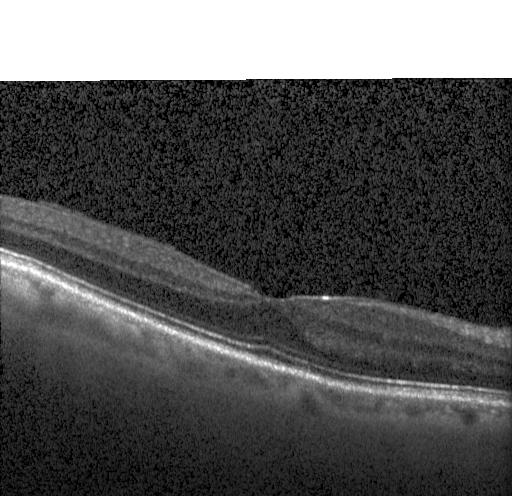

OCT line scan. Finding: no CNV, no DME, and no drusen.